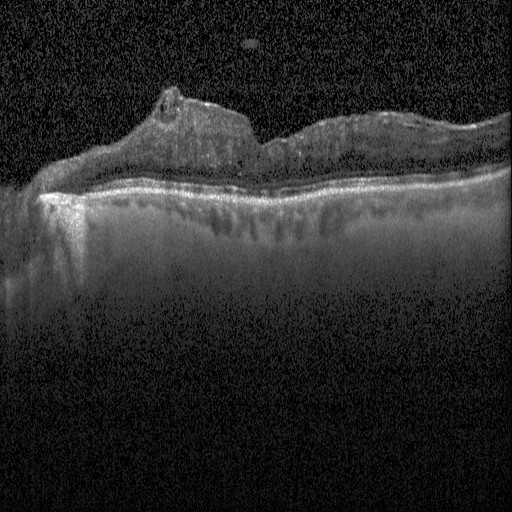

Retinal OCT cross-section. Centered on the fovea. Diagnosis: DME.